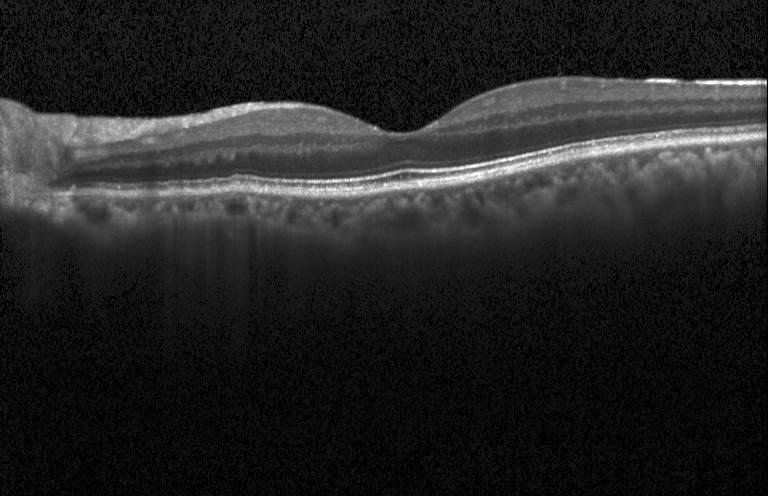 OCT B-scan, spectral-domain optical coherence tomography, fovea-centered.
Assessment: no evidence of choroidal neovascularization, diabetic macular edema, or drusen.